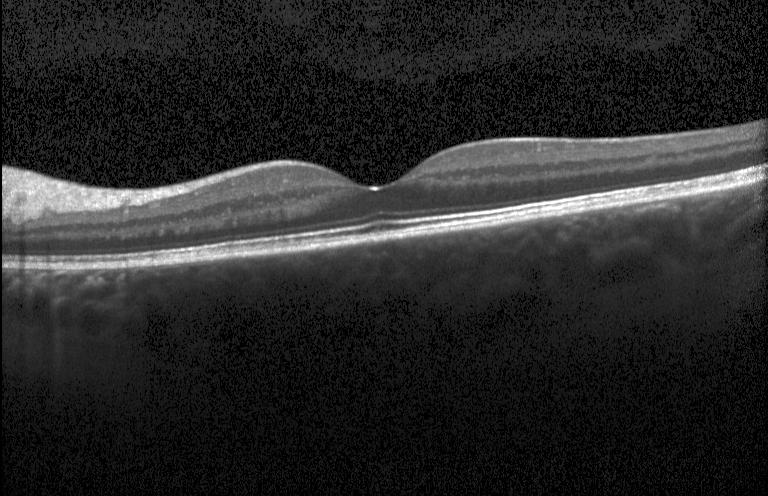

Retinal OCT B-scan — Finding: neither choroidal neovascularization, diabetic macular edema, nor drusen.